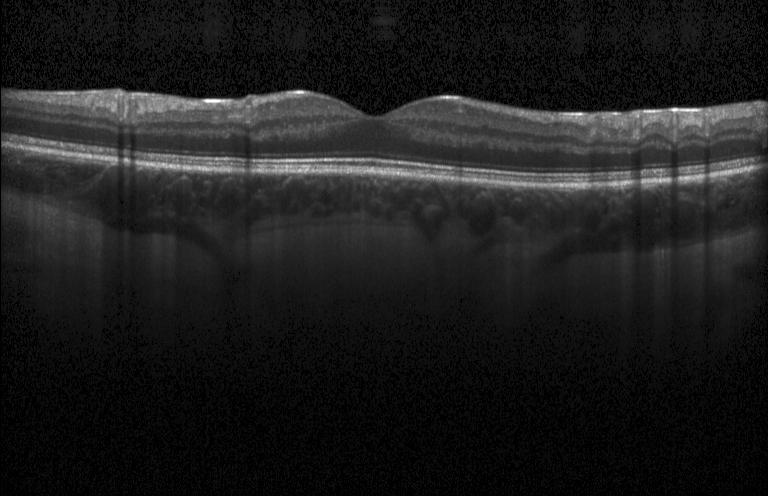

Macular scan, retinal OCT B-scan, spectral-domain optical coherence tomography, instrument: Heidelberg Spectralis. Finding: no choroidal neovascularization, diabetic macular edema, or drusen.